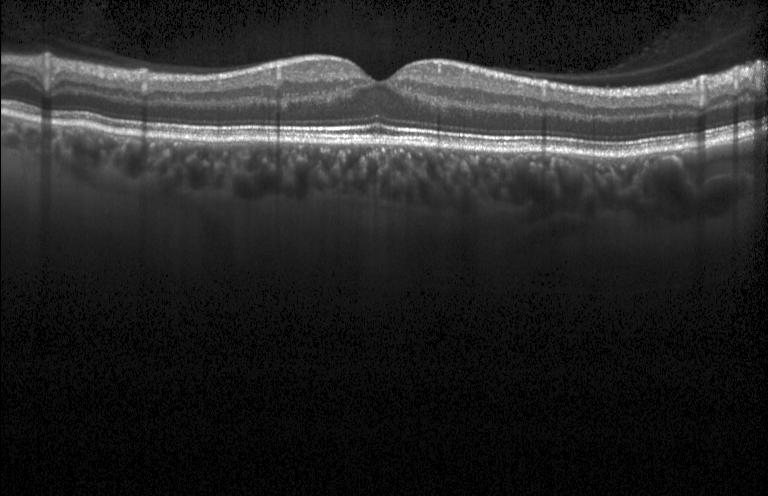 Retinal OCT B-scan; spectral-domain optical coherence tomography. Diagnosis: no choroidal neovascularization, diabetic macular edema, or drusen.